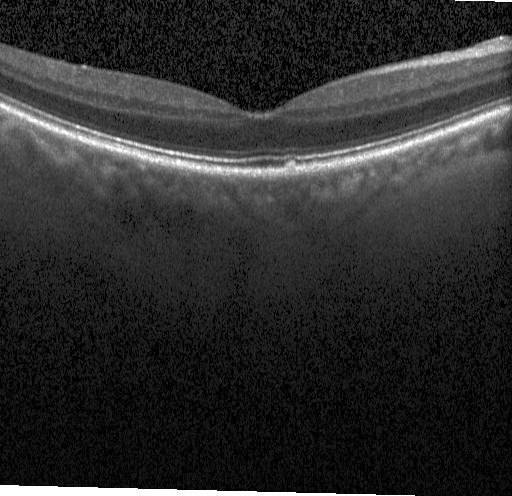

Through the macula; optical coherence tomography scan.
OCT finding: neither CNV, DME, nor drusen.